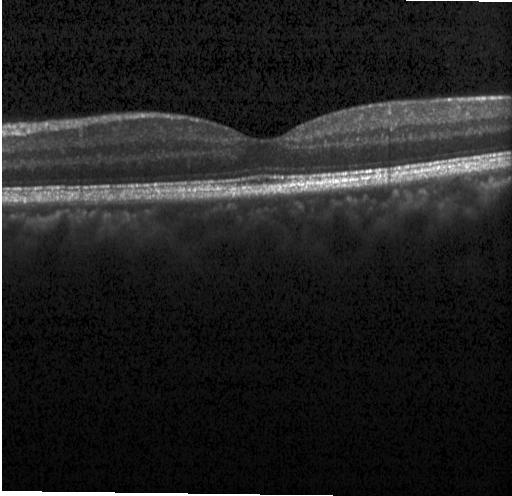 Retinal OCT B-scan
Assessment: no evidence of choroidal neovascularization, diabetic macular edema, or drusen.